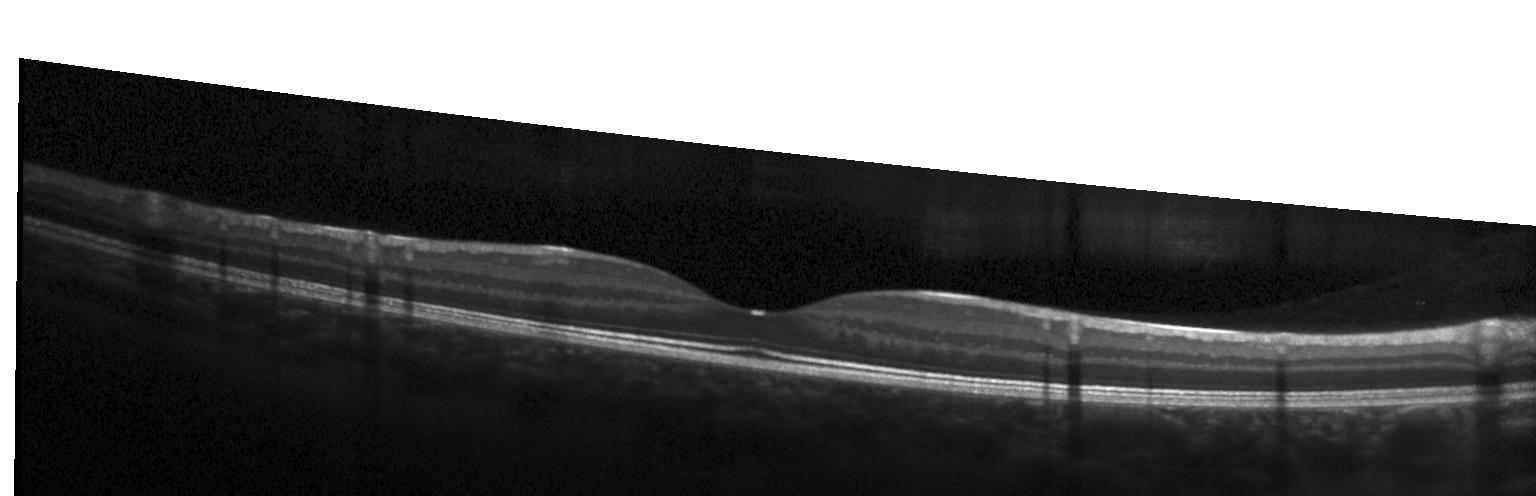

Macular OCT: neither CNV, DME, nor drusen.